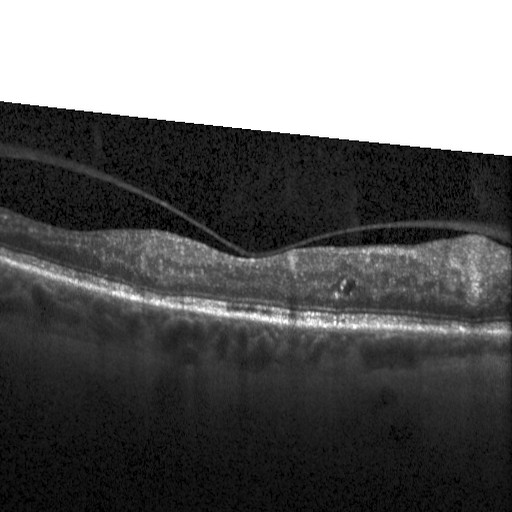

OCT B-scan — Diagnosis: diabetic macular edema (DME).